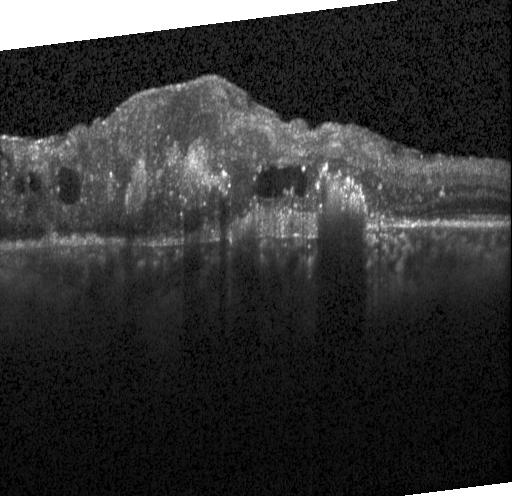
Finding: a choroidal neovascular membrane.